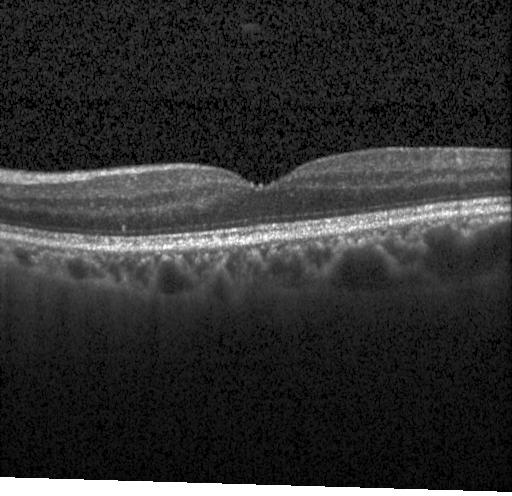
Optical coherence tomography B-scan, Heidelberg Spectralis, spectral-domain OCT, centered on the fovea. No evidence of choroidal neovascularization, diabetic macular edema, or drusen.